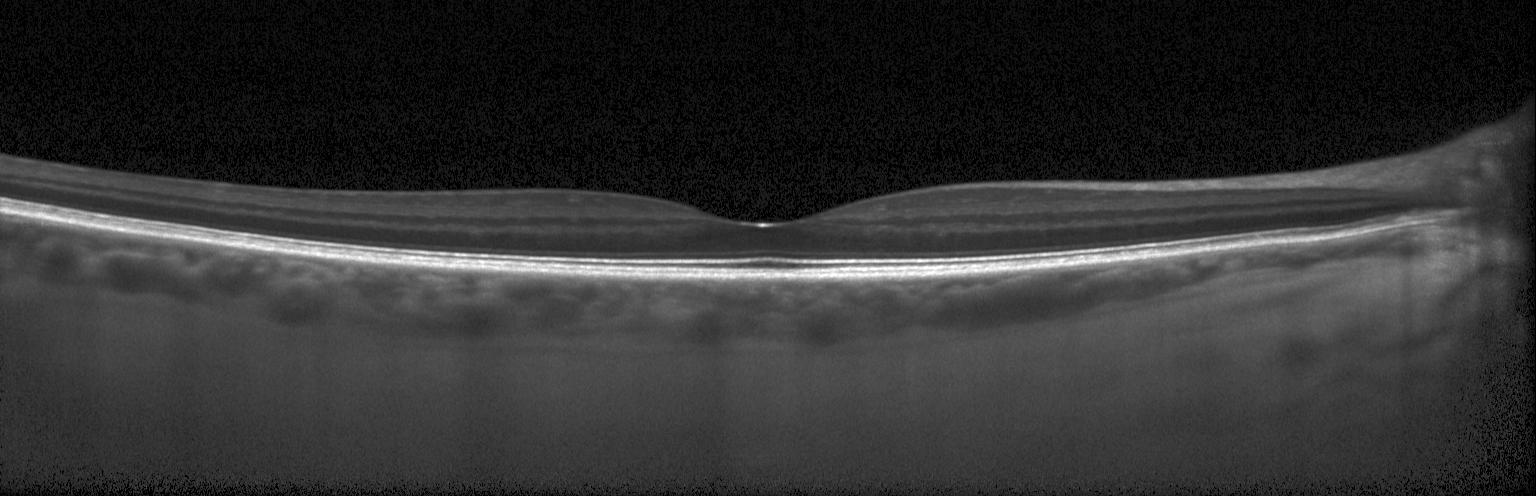
Macular scan, retinal OCT B-scan, instrument: Heidelberg Spectralis, spectral-domain optical coherence tomography.
Diagnosis: no CNV, DME, or drusen.